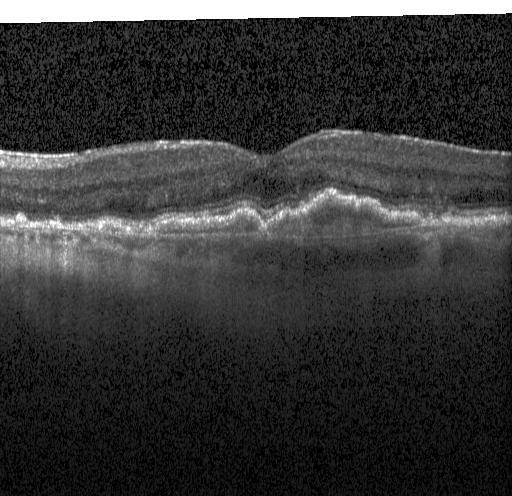 Finding: CNV.